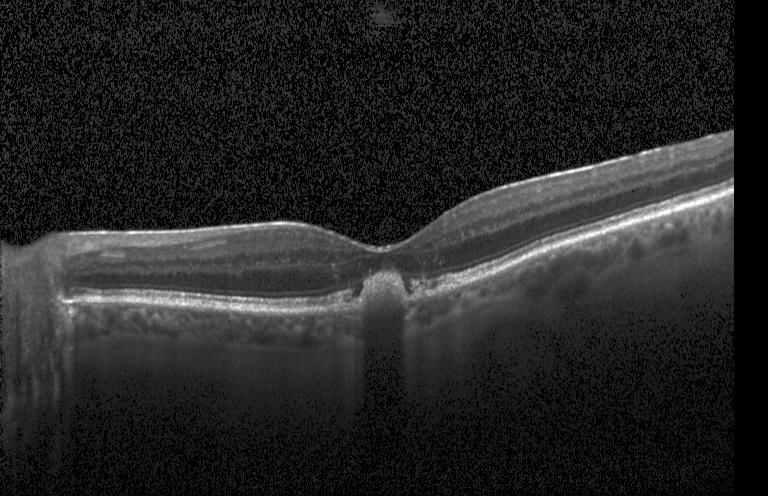
Macular OCT demonstrating a choroidal neovascular membrane.